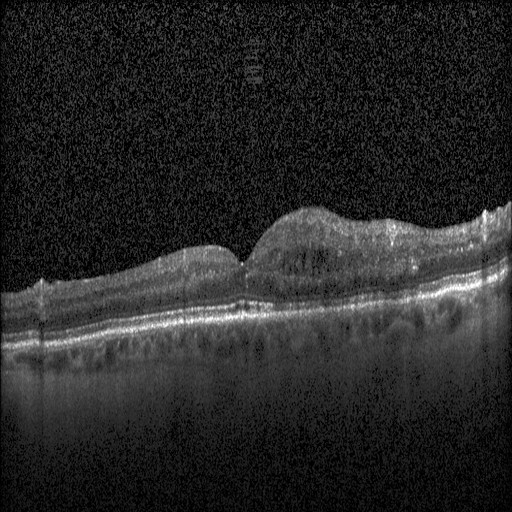

Optical coherence tomography B-scan, Heidelberg Spectralis OCT system — This B-scan demonstrates DME.